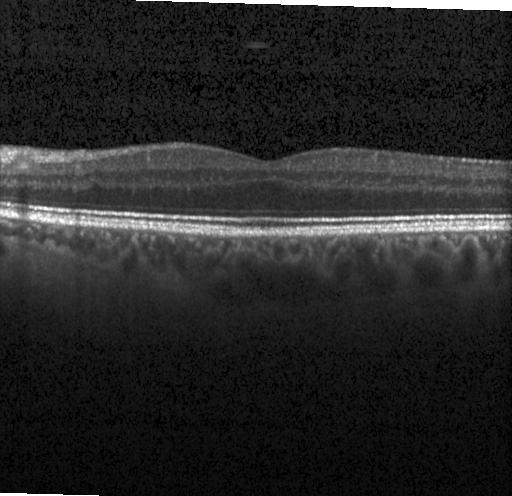
Fovea-centered. Retinal OCT cross-section. Acquired on a Heidelberg Spectralis. Neither choroidal neovascularization, diabetic macular edema, nor drusen.